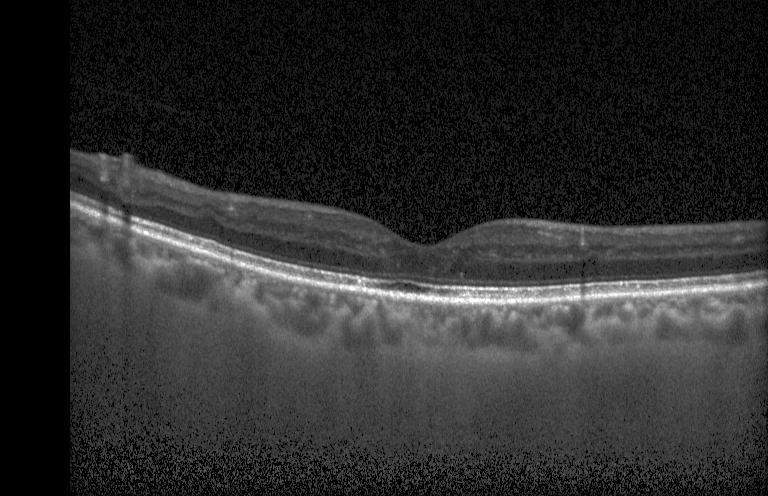 Impression: neither choroidal neovascularization, diabetic macular edema, nor drusen.